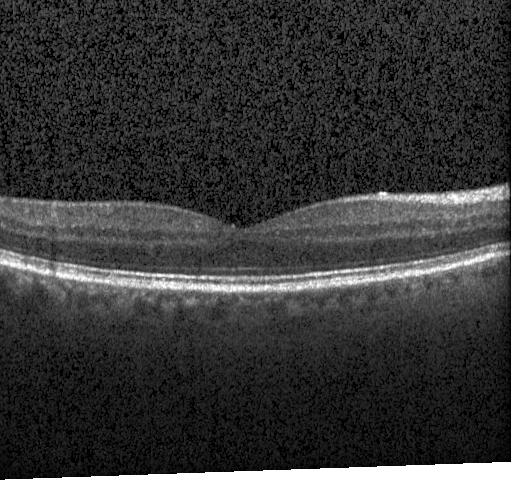
Macular OCT: no evidence of CNV, DME, or drusen.